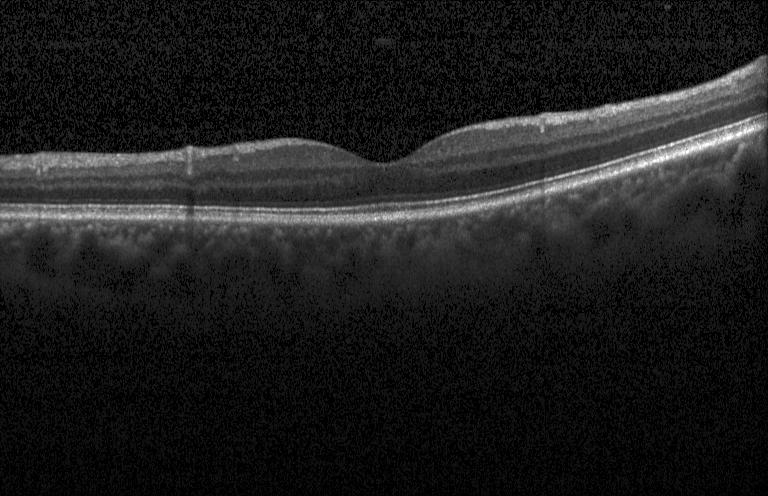
Retinal OCT cross-section · through the macula · spectral-domain optical coherence tomography. This B-scan demonstrates no evidence of CNV, DME, or drusen.